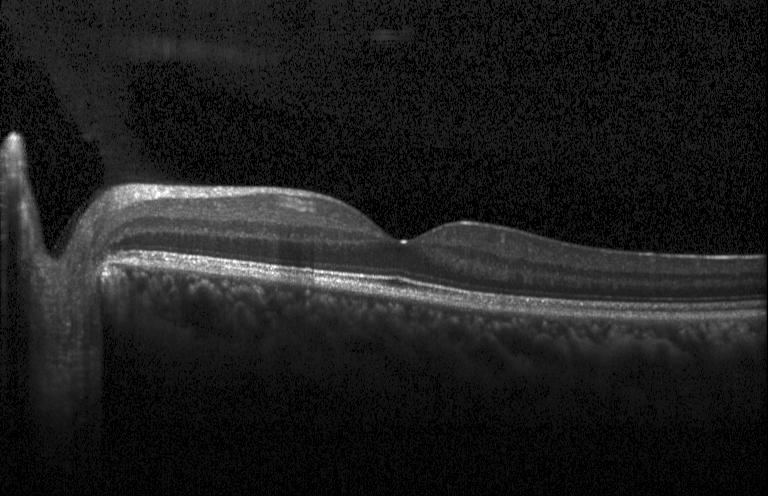
Retinal OCT B-scan; fovea-centered.
Finding: no evidence of CNV, DME, or drusen.